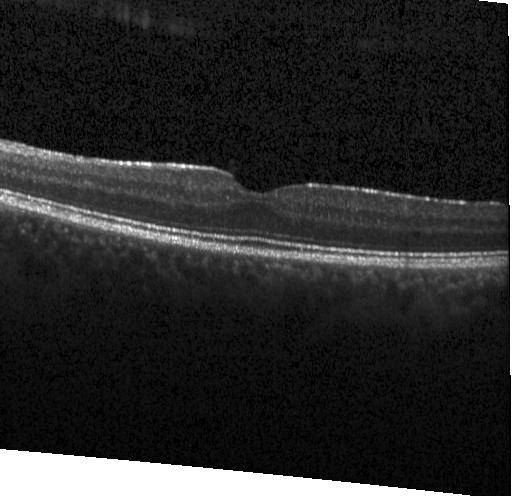

Diagnosis: no CNV, no DME, and no drusen.